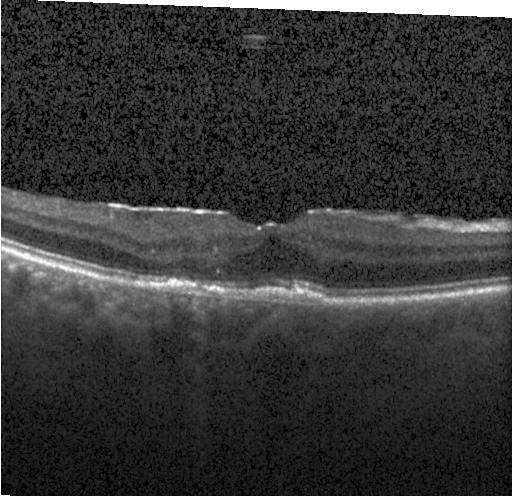
SD-OCT; optical coherence tomography scan; Heidelberg Spectralis
Impression: choroidal neovascularization (CNV).